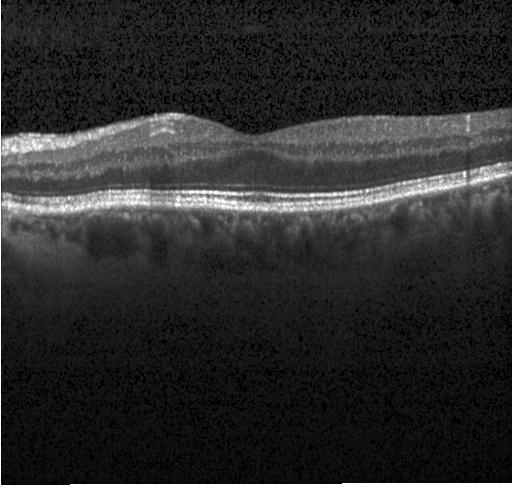

OCT line scan
The scan shows no evidence of choroidal neovascularization, diabetic macular edema, or drusen.